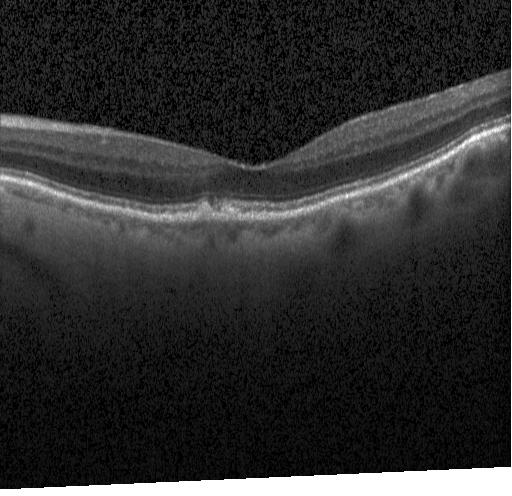 Heidelberg Spectralis OCT system, horizontal scan through the fovea, optical coherence tomography scan, SD-OCT. Finding: sub-RPE drusenoid deposits.